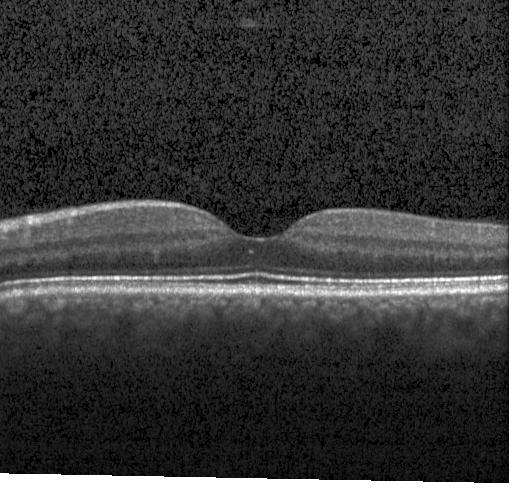 OCT line scan; through the macula; instrument: Heidelberg Spectralis
Finding: no choroidal neovascularization, diabetic macular edema, or drusen.